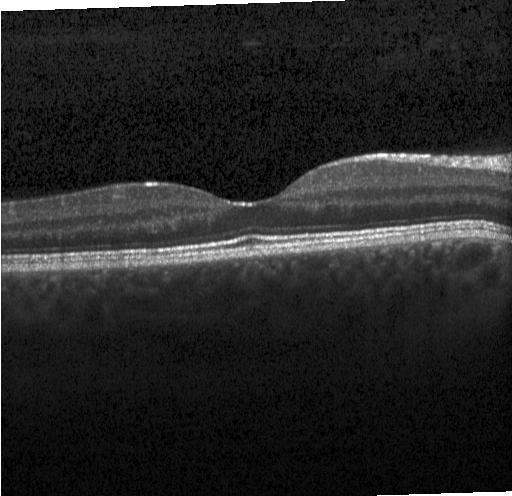 Acquired on a Heidelberg Spectralis, optical coherence tomography scan. Assessment: neither choroidal neovascularization, diabetic macular edema, nor drusen.